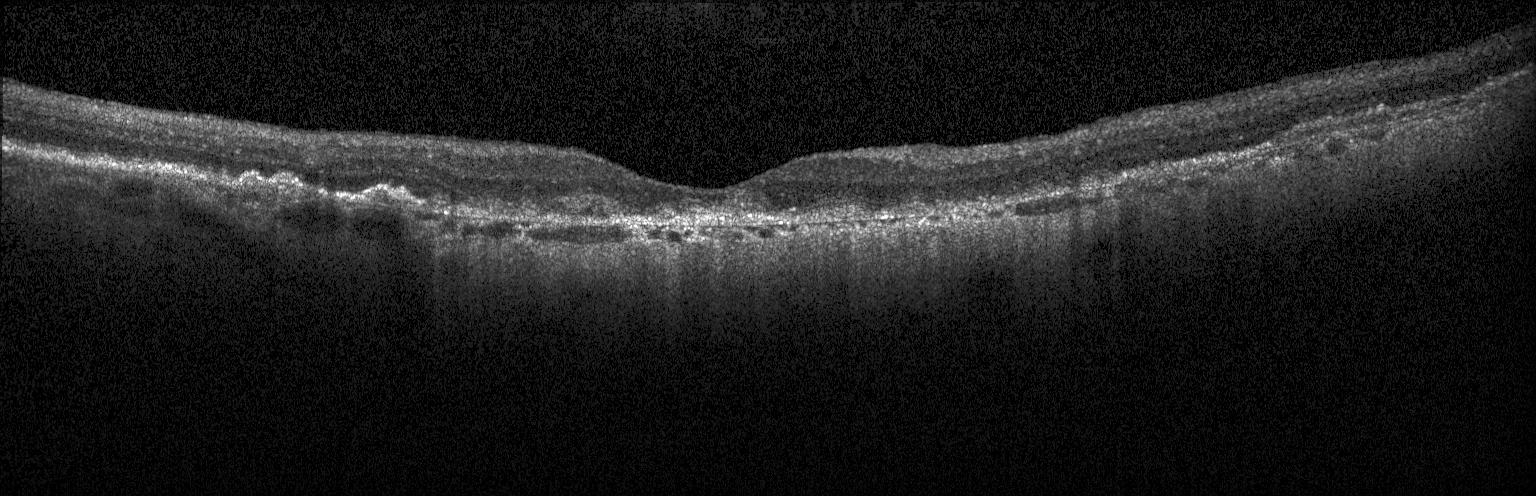

Finding: a choroidal neovascular membrane.